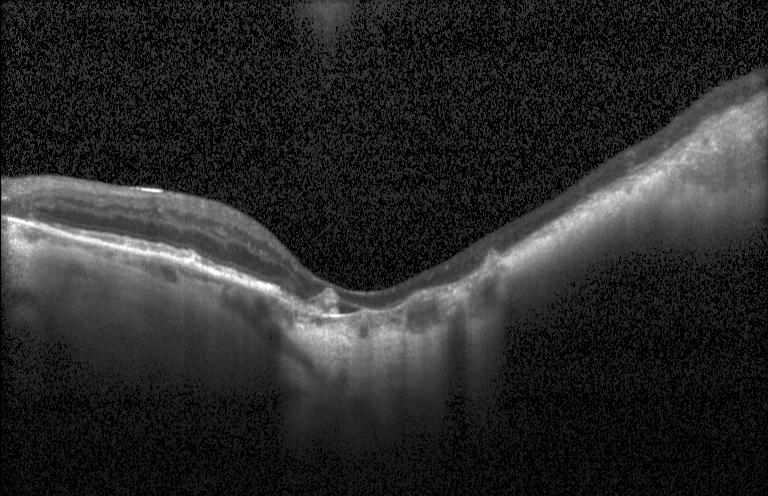

Through the macula; optical coherence tomography B-scan
Diagnosis: choroidal neovascularization (CNV).